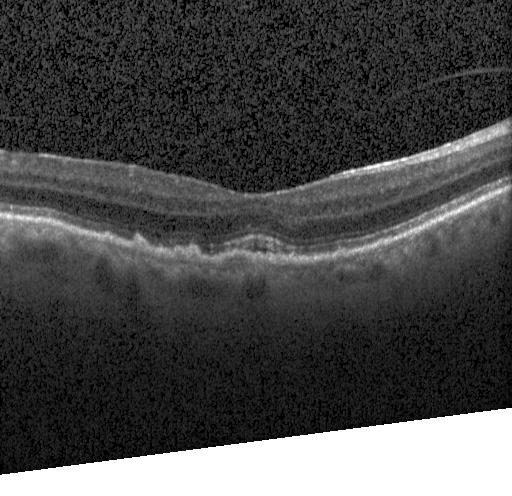 Retinal OCT cross-section
Assessment: choroidal neovascularization (CNV).